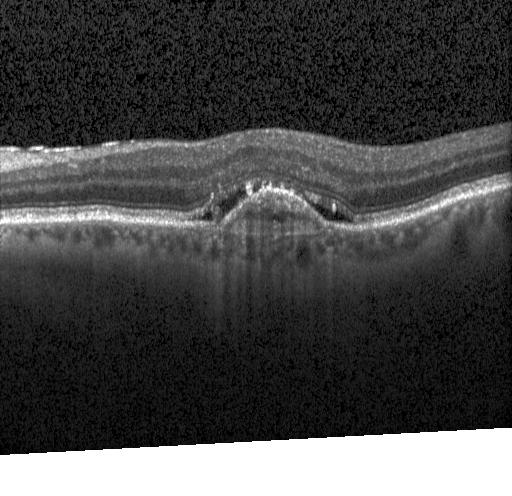

Retinal OCT cross-section. Horizontal scan through the fovea. Acquired on a Heidelberg Spectralis.
Diagnosis: a choroidal neovascular membrane.